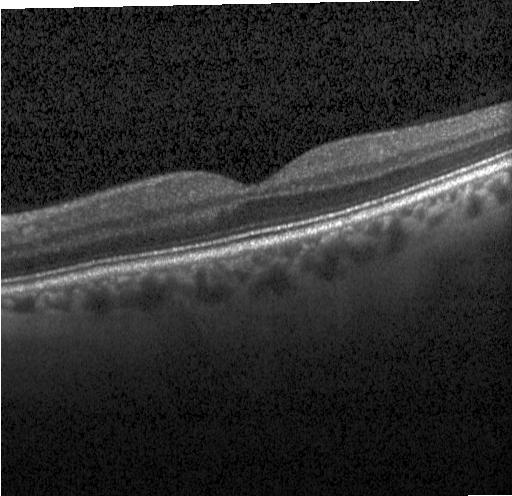 Finding: no CNV, no DME, and no drusen.